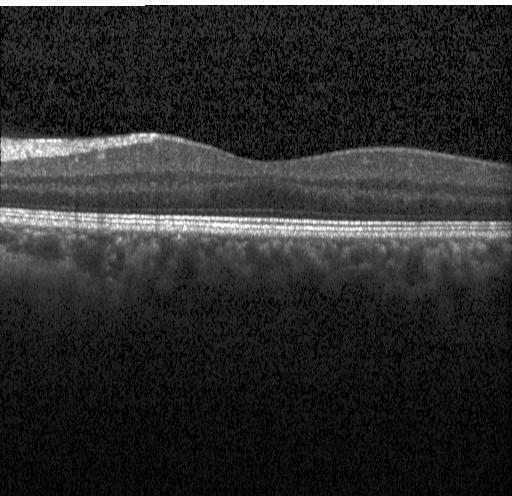 Retinal OCT cross-section
Dx: neither choroidal neovascularization, diabetic macular edema, nor drusen.